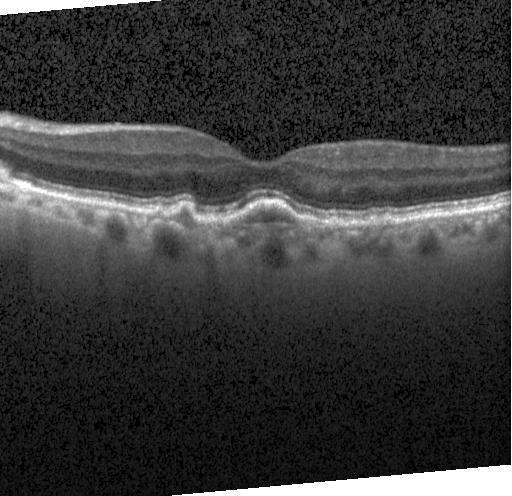

Optical coherence tomography scan; SD-OCT
A choroidal neovascular membrane.